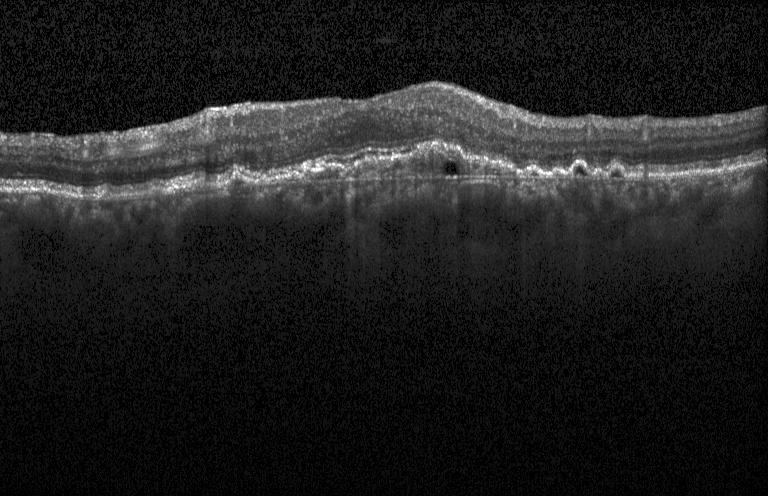
Retinal OCT cross-section showing choroidal neovascularization.